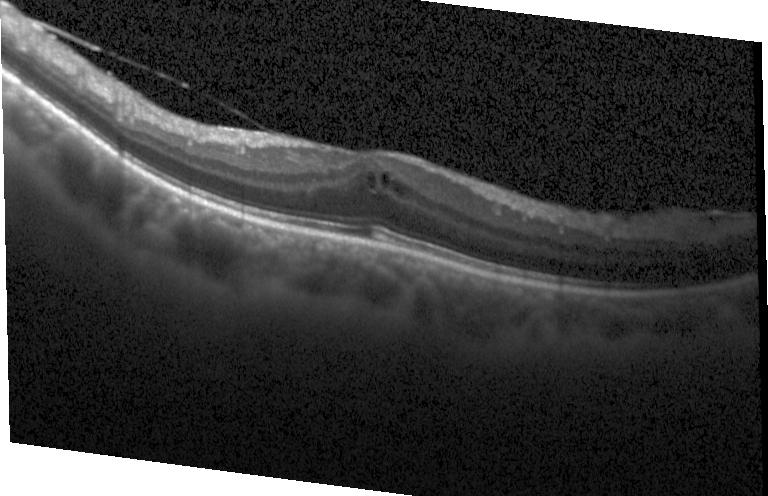
Diagnosis: diabetic macular edema (DME).